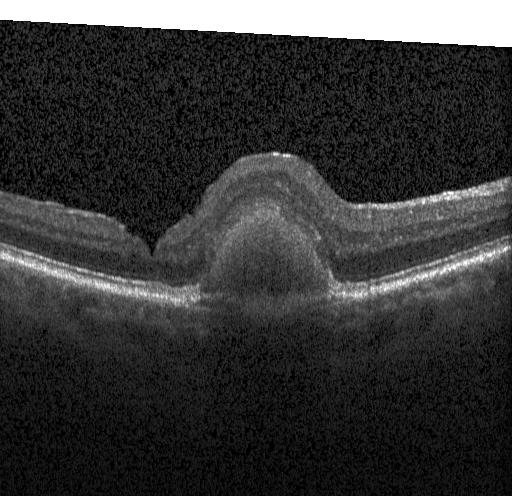 OCT line scan, spectral-domain OCT — This B-scan demonstrates a choroidal neovascular membrane.